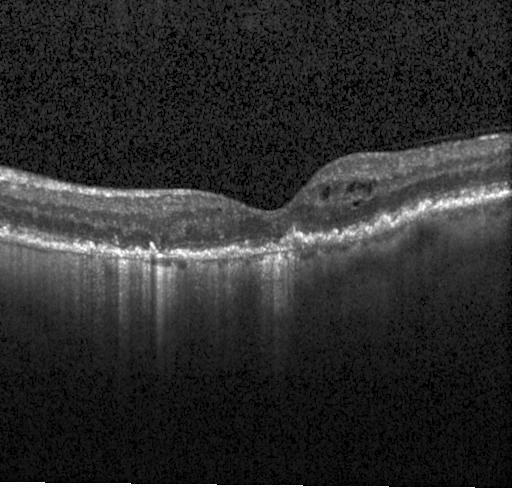

OCT finding: a choroidal neovascular membrane.